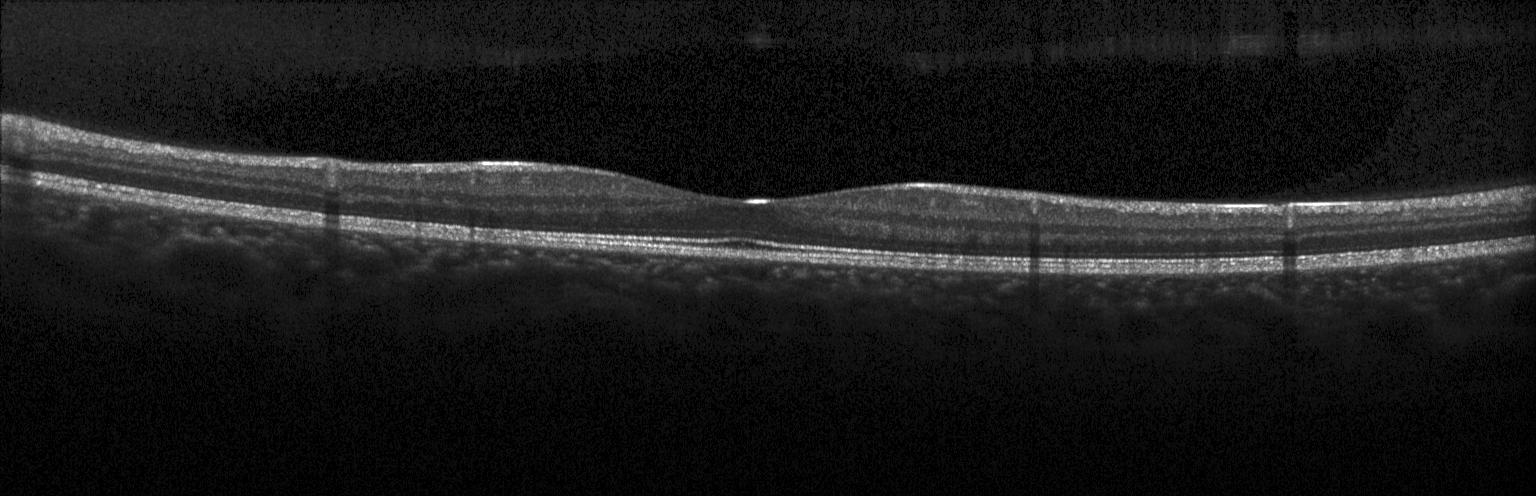 SD-OCT. Macular scan. Instrument: Heidelberg Spectralis. Optical coherence tomography B-scan
Dx: no CNV, DME, or drusen.